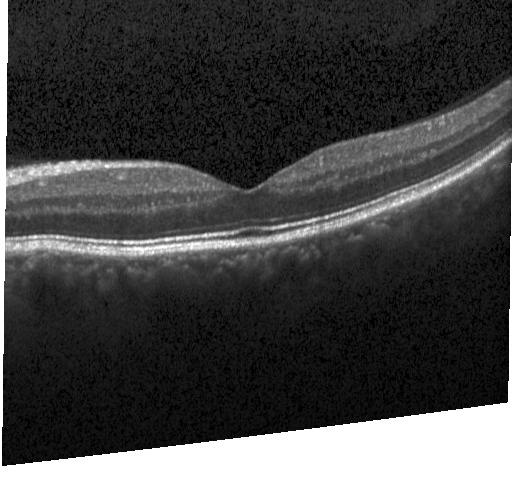
Macular scan; instrument: Heidelberg Spectralis; retinal OCT B-scan; SD-OCT — Impression: no CNV, no DME, and no drusen.